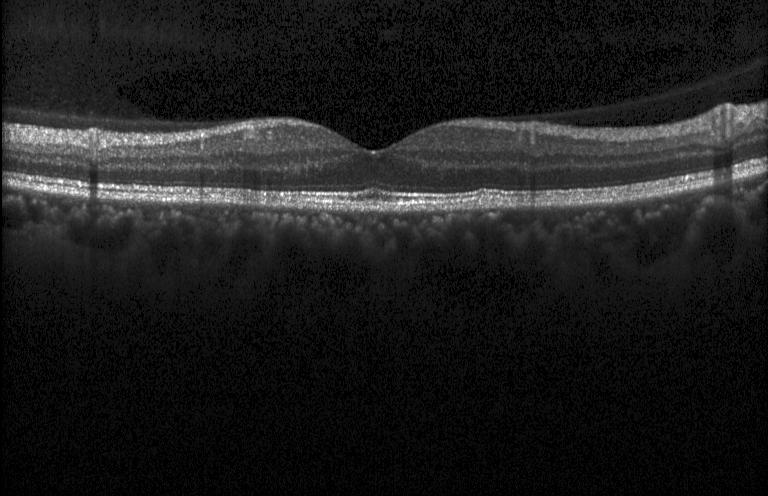 Finding: no choroidal neovascularization, diabetic macular edema, or drusen.